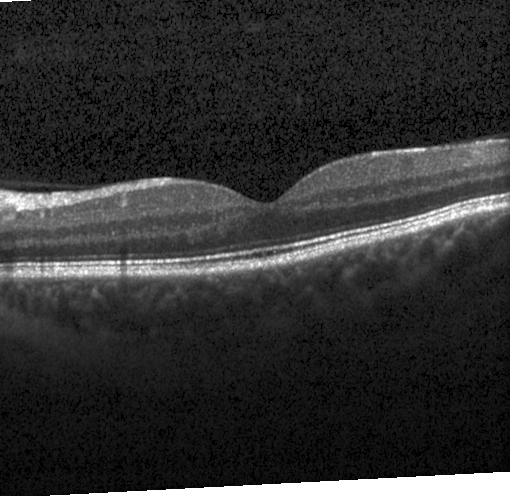

Finding: no choroidal neovascularization, diabetic macular edema, or drusen.